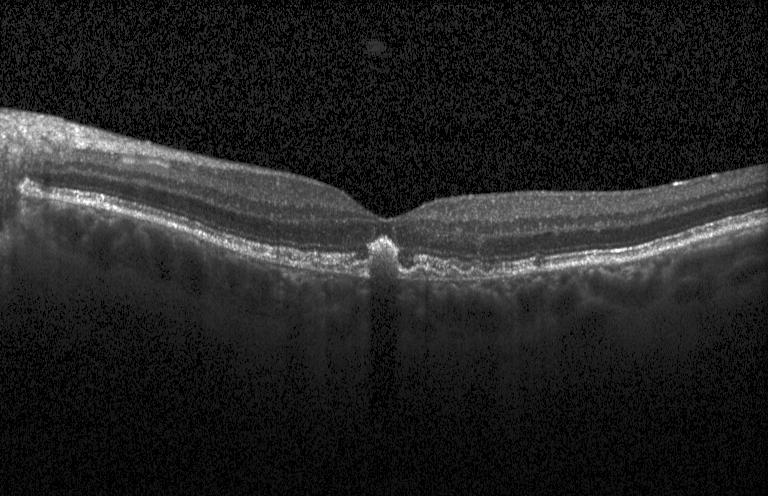

Optical coherence tomography B-scan. Macular OCT: CNV.